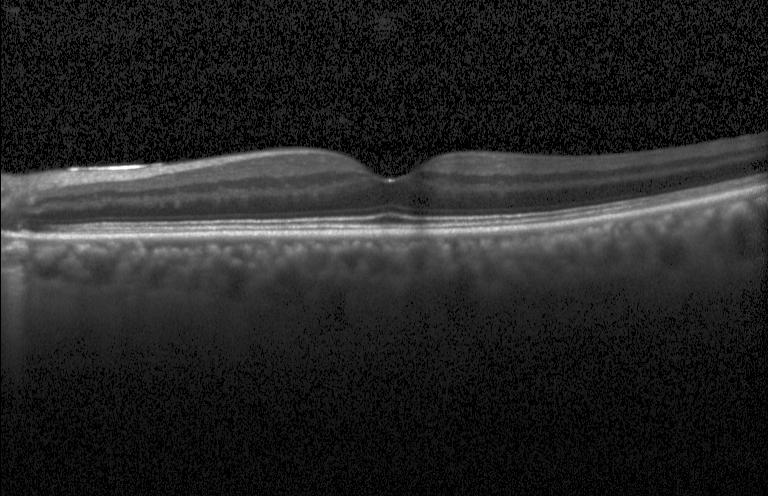 Through the macula; retinal OCT cross-section; SD-OCT. Finding: no choroidal neovascularization, diabetic macular edema, or drusen.